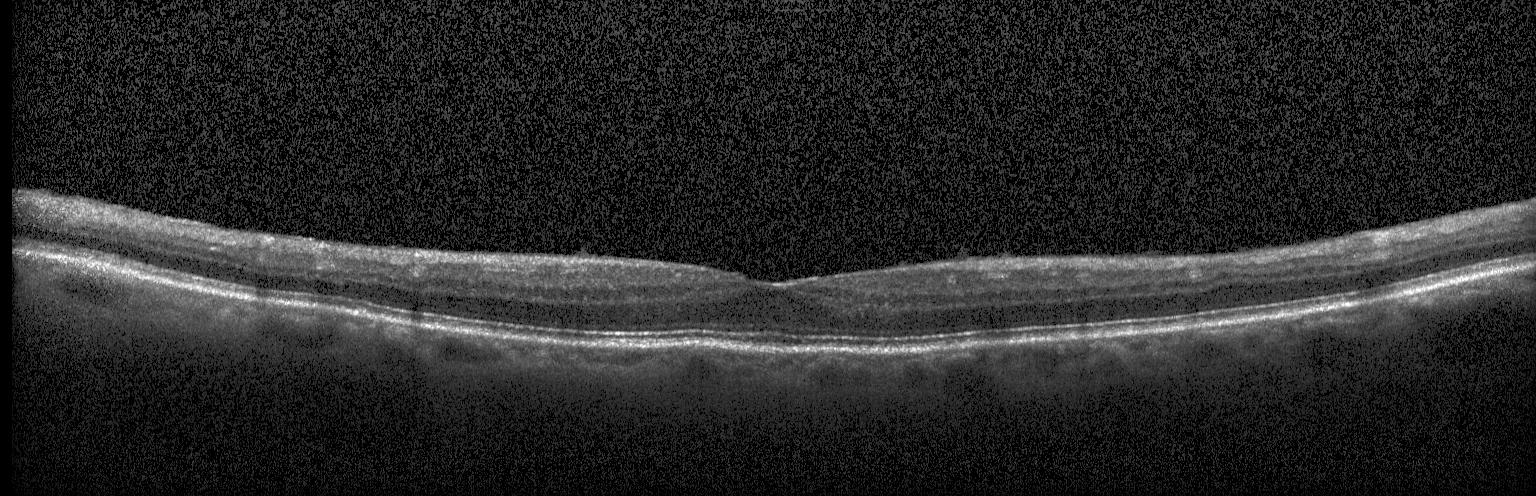

Macular OCT demonstrating no evidence of choroidal neovascularization, diabetic macular edema, or drusen.